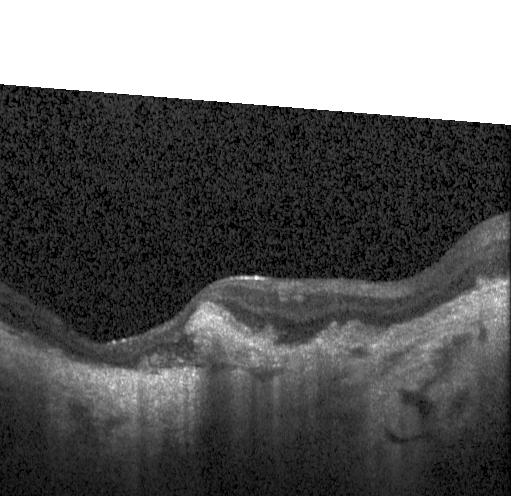
Instrument: Heidelberg Spectralis; optical coherence tomography B-scan; spectral-domain optical coherence tomography; centered on the fovea.
Impression: a choroidal neovascular membrane.